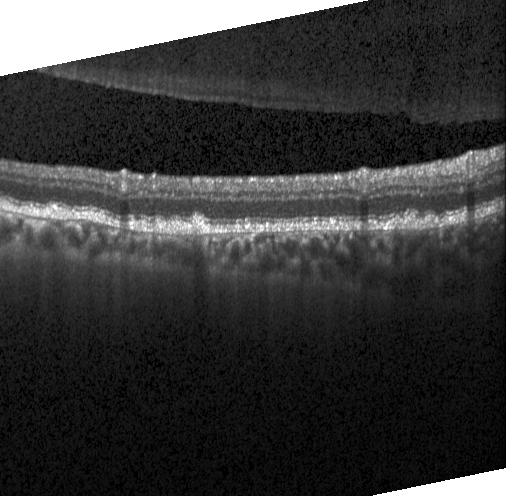 Optical coherence tomography B-scan · Heidelberg Spectralis OCT system · spectral-domain OCT · through the macula
Finding: sub-RPE drusenoid deposits.